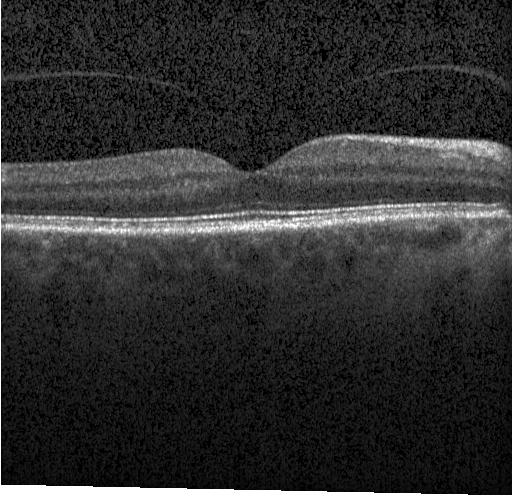
Retinal OCT B-scan, acquired on a Heidelberg Spectralis, through the macula, SD-OCT.
Finding: no CNV, no DME, and no drusen.